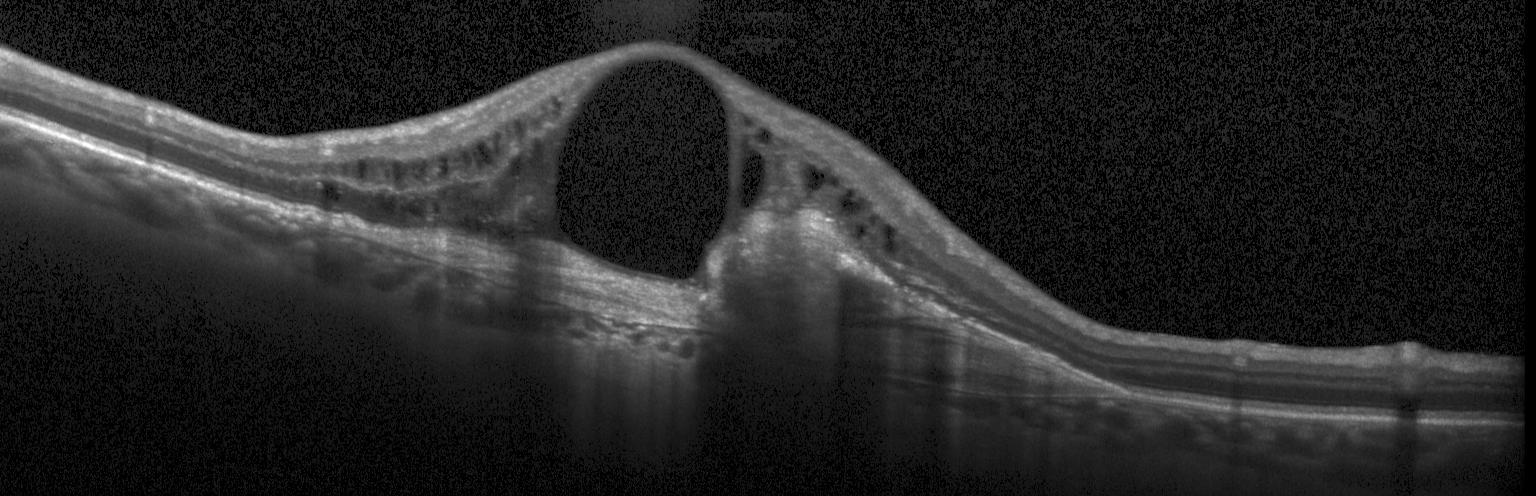 SD-OCT. Optical coherence tomography scan. Acquired on a Heidelberg Spectralis. Dx: a choroidal neovascular membrane.